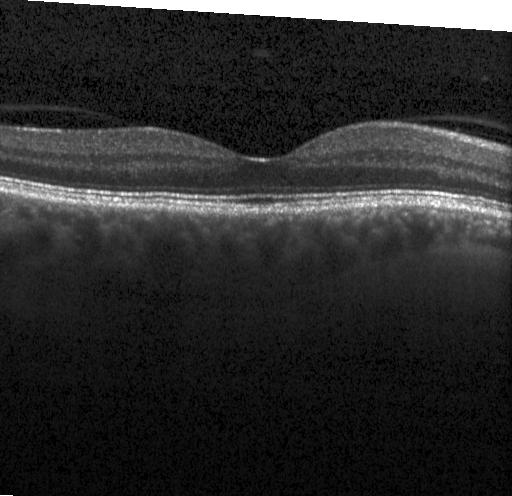
Finding: no evidence of choroidal neovascularization, diabetic macular edema, or drusen.